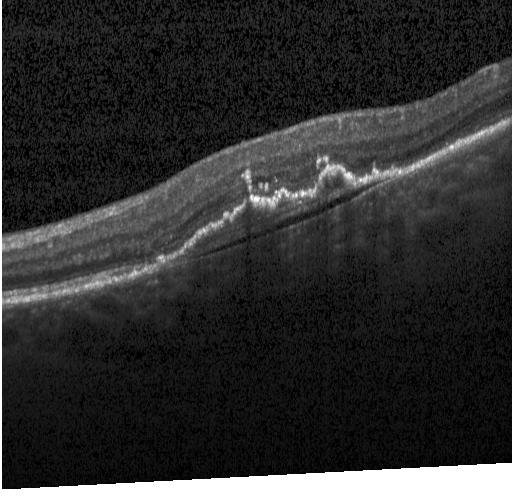

Retinal OCT cross-section · SD-OCT
Impression: choroidal neovascularization.